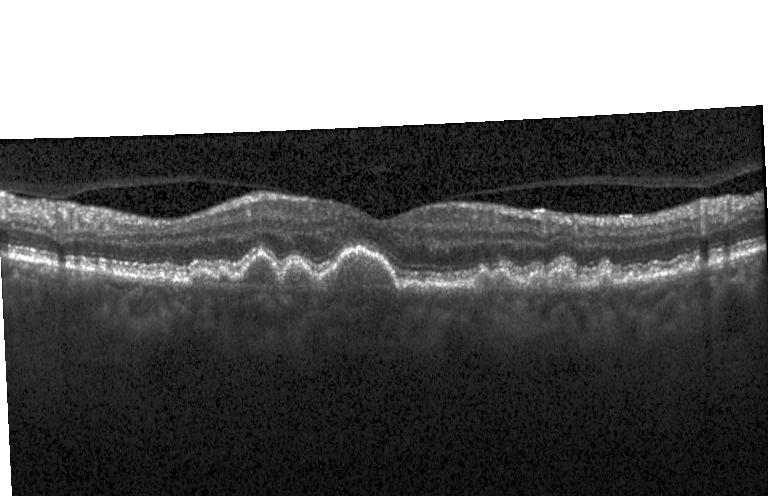

Macular scan. OCT line scan. Spectral-domain OCT — This B-scan demonstrates sub-RPE drusenoid deposits.